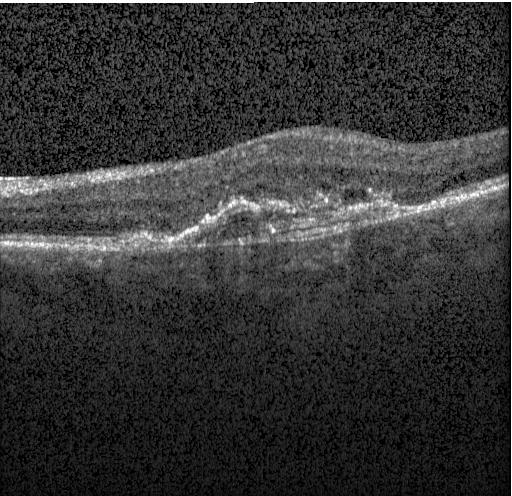
OCT B-scan · Heidelberg Spectralis OCT system — Macular OCT: choroidal neovascularization.